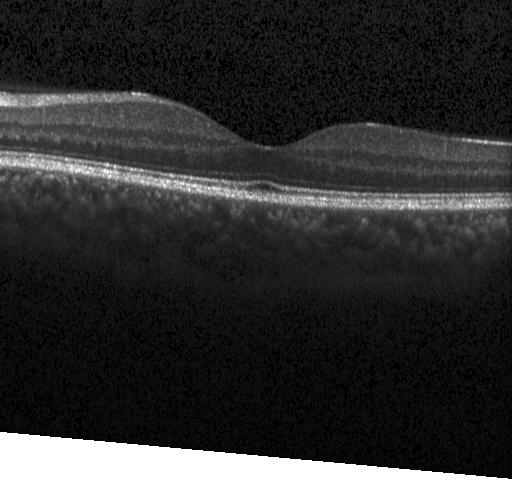 Macular OCT: neither choroidal neovascularization, diabetic macular edema, nor drusen.